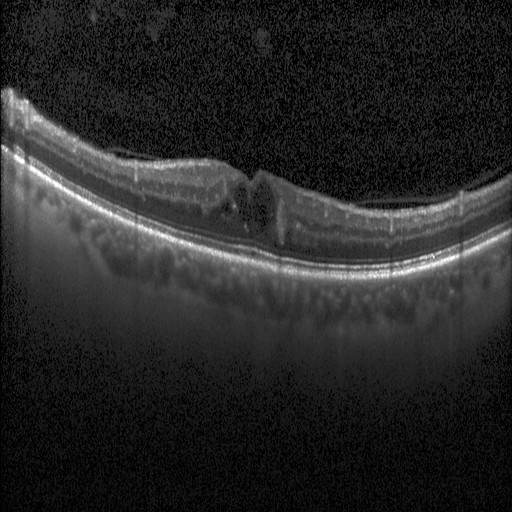

Retinal OCT cross-section. Centered on the fovea. Heidelberg Spectralis OCT system — The scan shows DME.